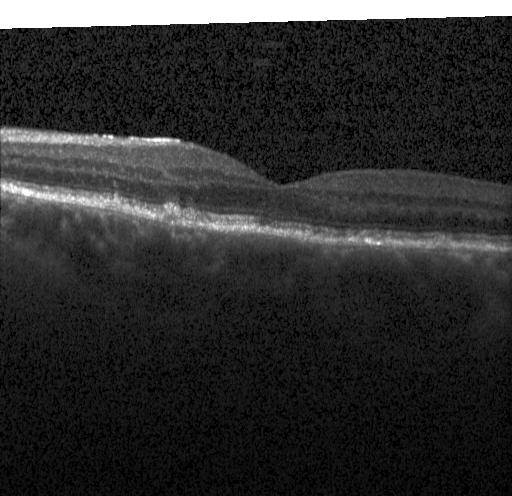 OCT line scan — Diagnosis: drusen.